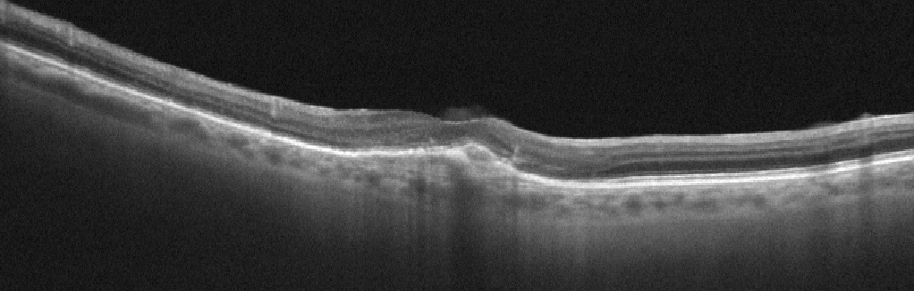 Optovue Avanti RTVue XR, OCT line scan — OCT finding: AMD.